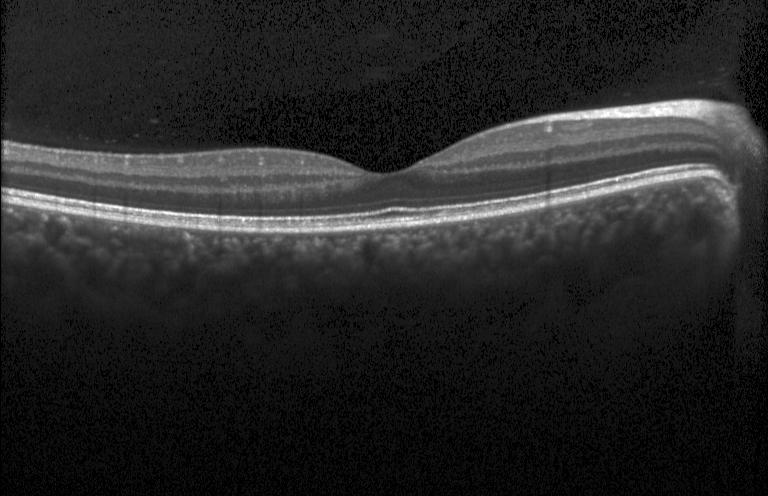 Spectral-domain OCT · optical coherence tomography scan. Impression: no evidence of choroidal neovascularization, diabetic macular edema, or drusen.